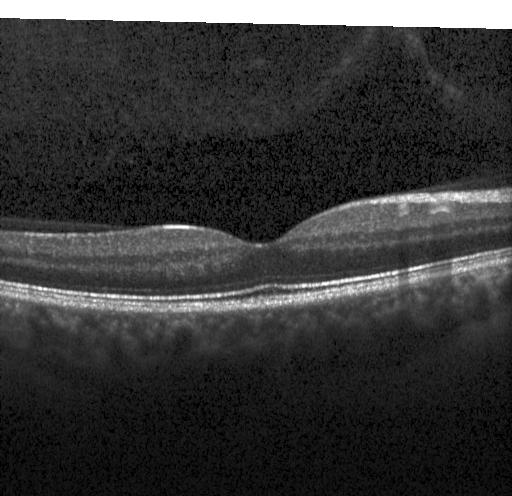

OCT line scan. Spectral-domain OCT. Macular scan. Diagnosis: neither CNV, DME, nor drusen.